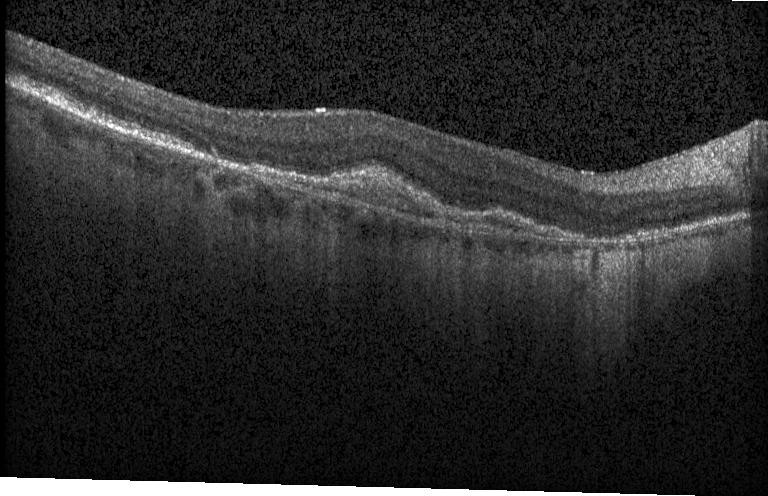 Fovea-centered · spectral-domain OCT · instrument: Heidelberg Spectralis · optical coherence tomography scan — CNV.